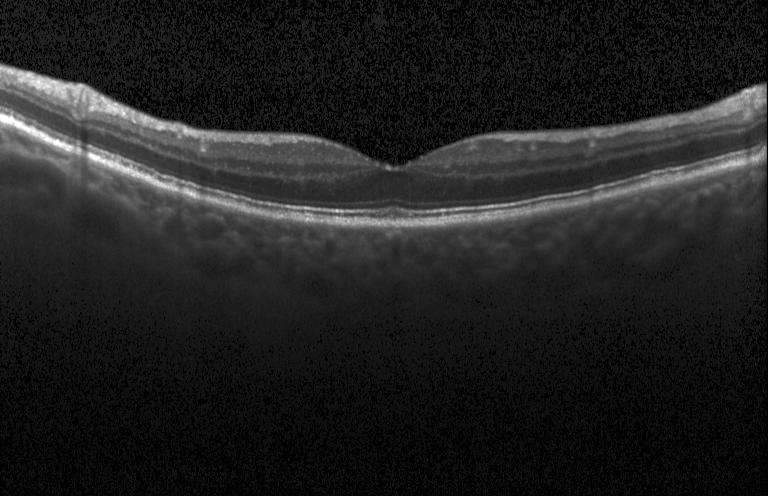

Diagnosis: no evidence of choroidal neovascularization, diabetic macular edema, or drusen.